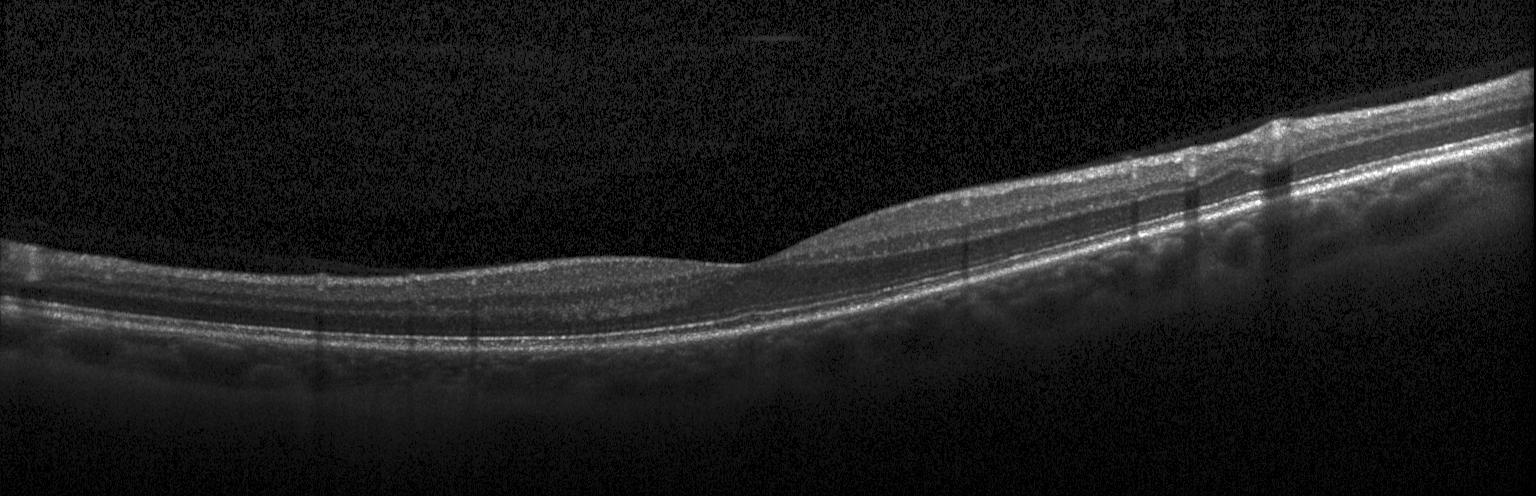
Optical coherence tomography scan. Heidelberg Spectralis OCT system. Spectral-domain optical coherence tomography. Through the macula. Diagnosis: no CNV, DME, or drusen.